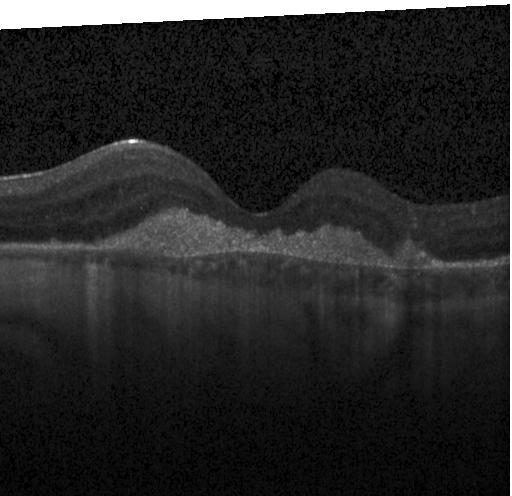

Diagnosis: choroidal neovascularization (CNV).